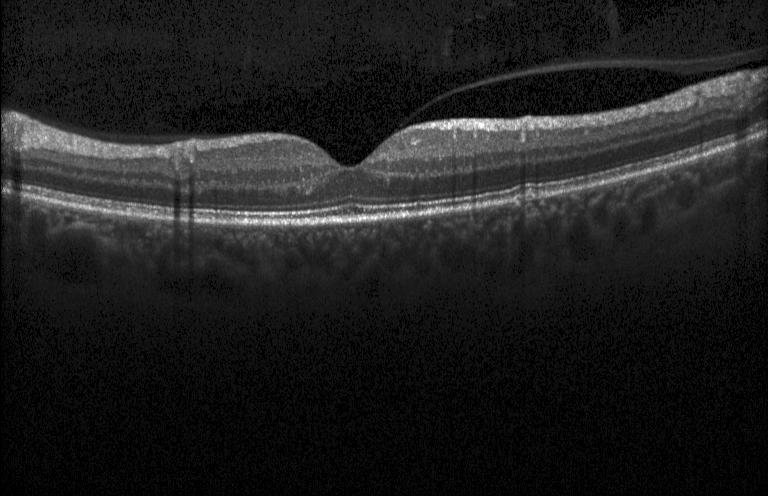

OCT scan showing neither choroidal neovascularization, diabetic macular edema, nor drusen.